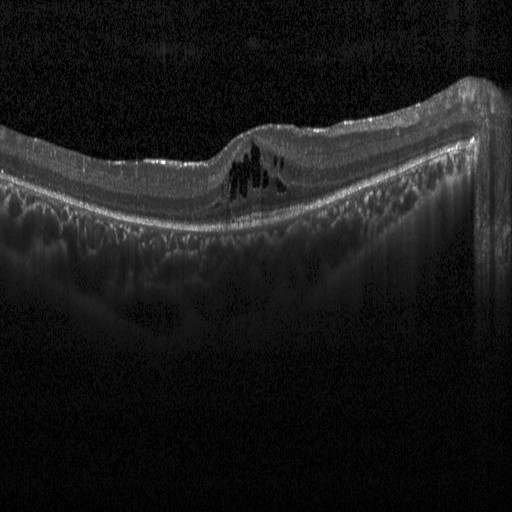
Impression: diabetic macular edema (DME).